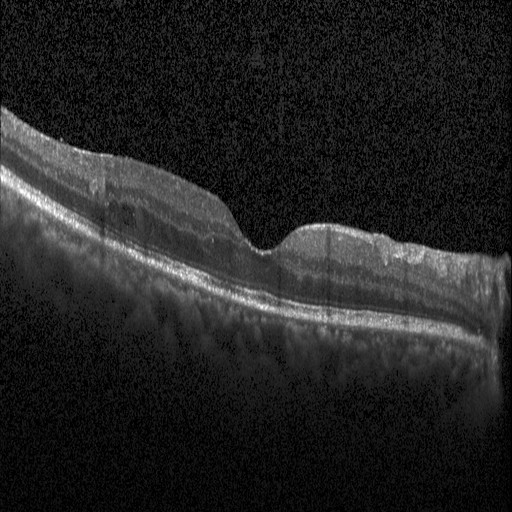

Optical coherence tomography scan. Diabetic macular edema.